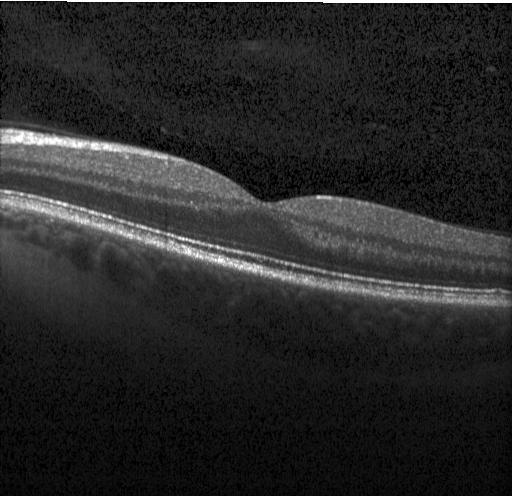
Optical coherence tomography scan. This B-scan demonstrates neither choroidal neovascularization, diabetic macular edema, nor drusen.